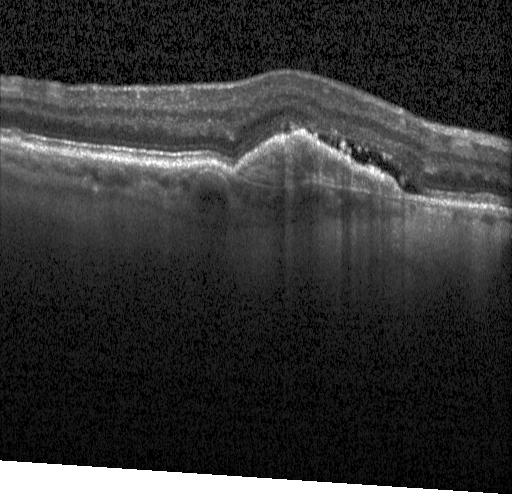

Optical coherence tomography scan · SD-OCT · horizontal scan through the fovea — Impression: a choroidal neovascular membrane.